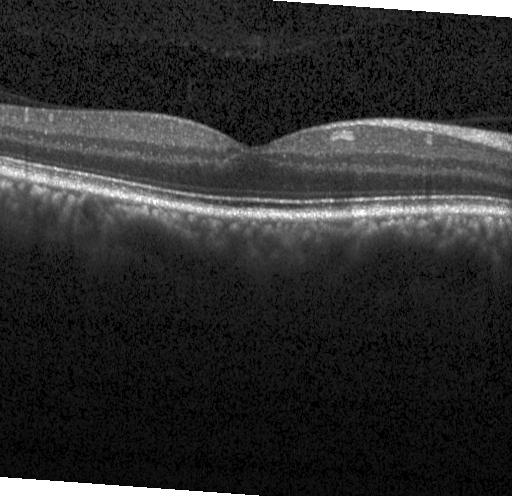 Optical coherence tomography B-scan
Finding: no choroidal neovascularization, diabetic macular edema, or drusen.